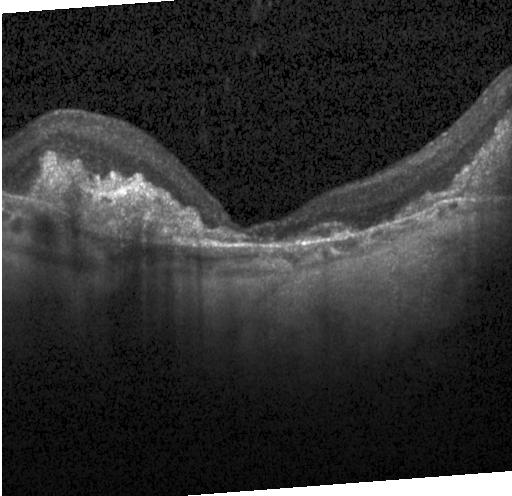

Optical coherence tomography scan, SD-OCT. Diagnosis: choroidal neovascularization.